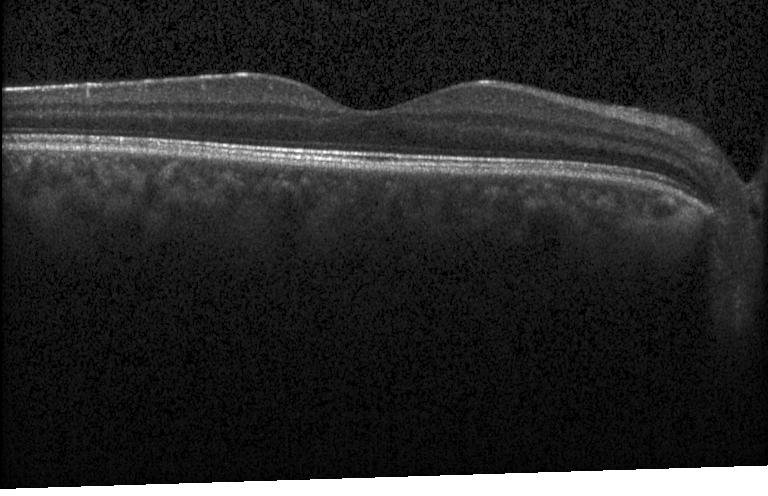 Diagnosis: no evidence of choroidal neovascularization, diabetic macular edema, or drusen.